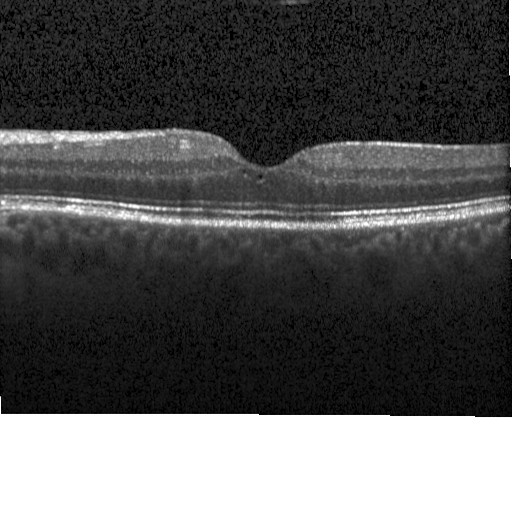
OCT finding: diabetic macular edema (DME).